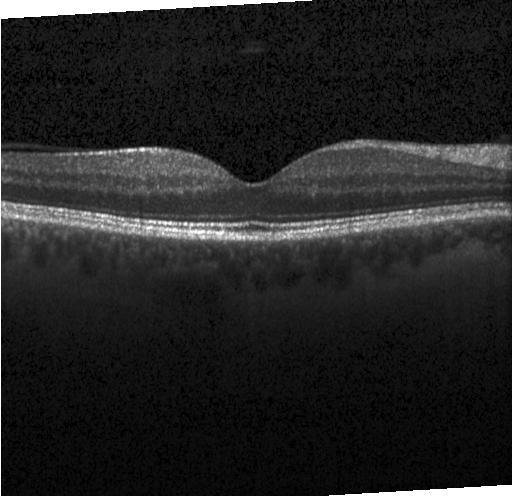
Fovea-centered, OCT line scan, spectral-domain optical coherence tomography
Diagnosis: no evidence of choroidal neovascularization, diabetic macular edema, or drusen.